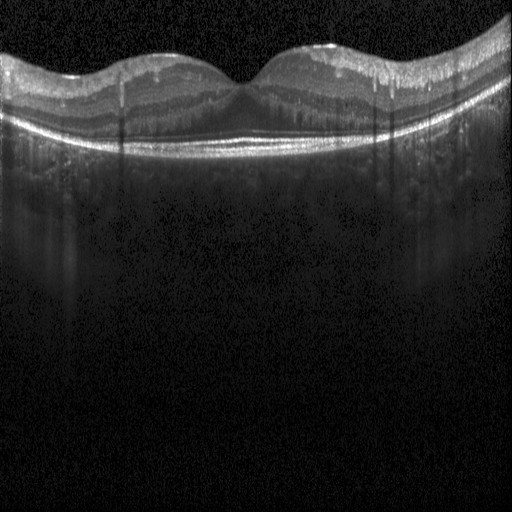
Optical coherence tomography B-scan · through the macula.
Diagnosis: diabetic macular edema (DME).